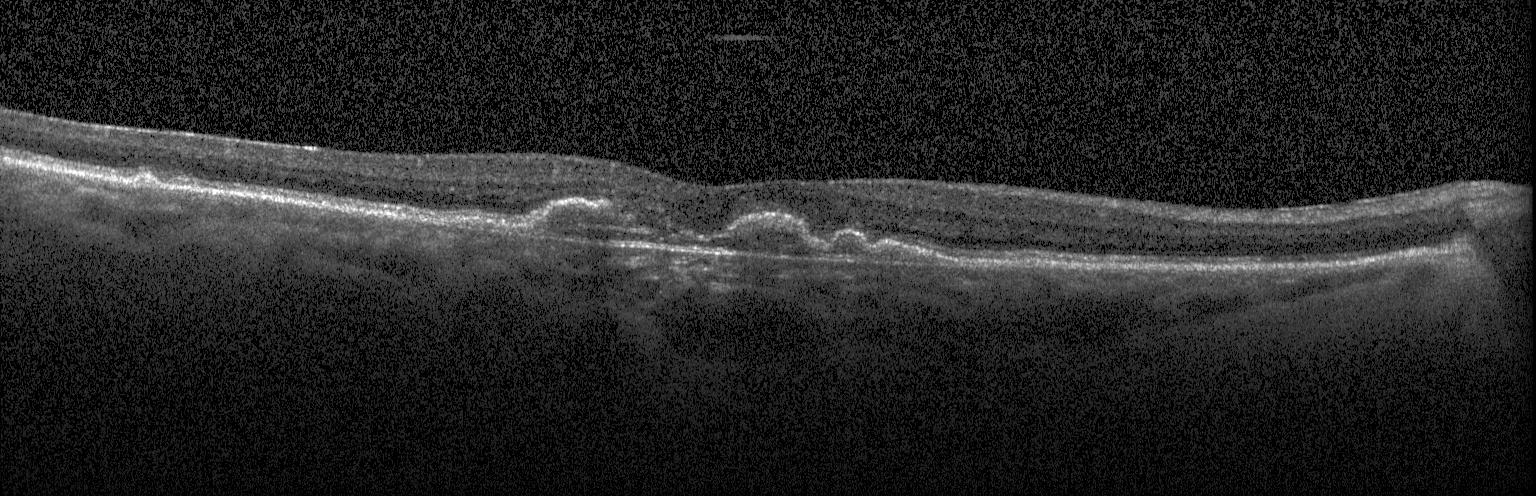

Horizontal scan through the fovea. OCT B-scan
Assessment: a choroidal neovascular membrane.